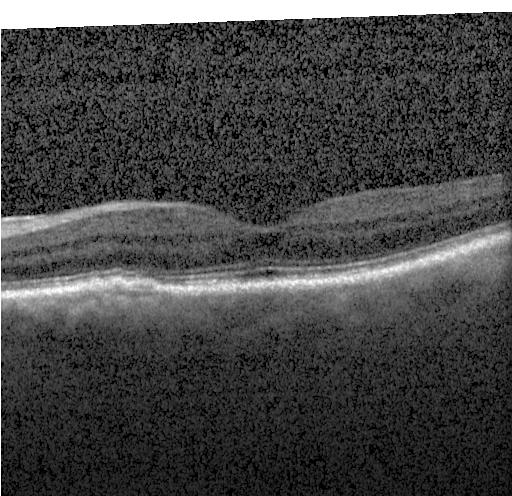 Fovea-centered. OCT line scan. SD-OCT. Instrument: Heidelberg Spectralis
This B-scan demonstrates multiple drusen.